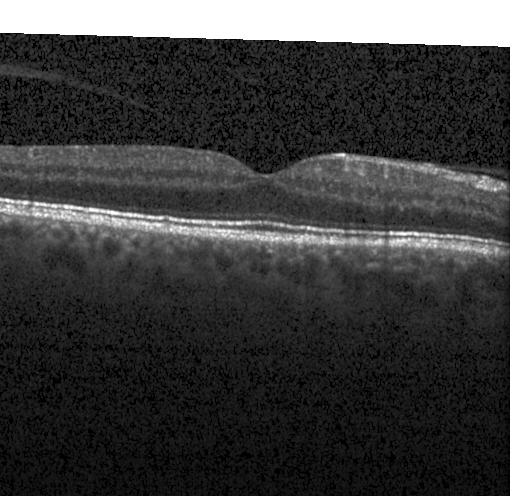 Centered on the fovea. Retinal OCT cross-section
Diagnosis: neither choroidal neovascularization, diabetic macular edema, nor drusen.